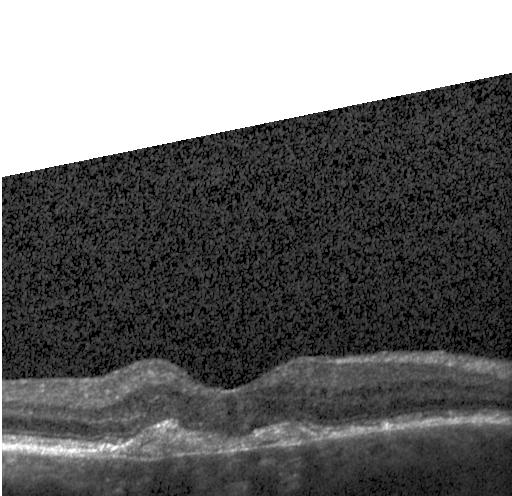
OCT line scan.
Finding: a choroidal neovascular membrane.